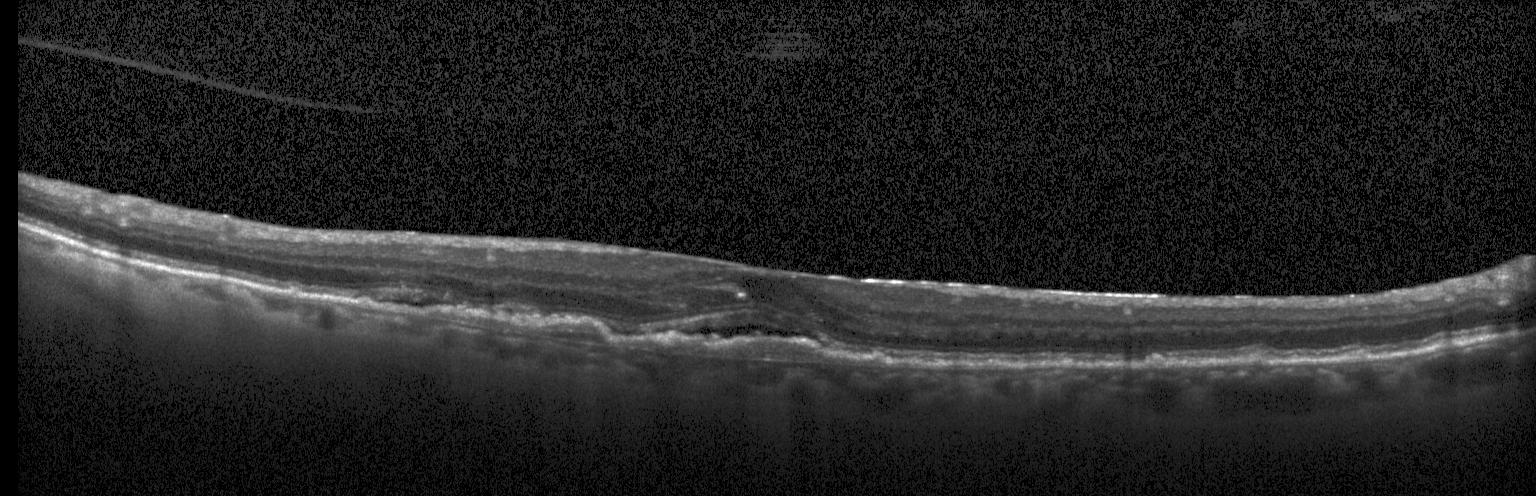
Retinal OCT cross-section showing a choroidal neovascular membrane.